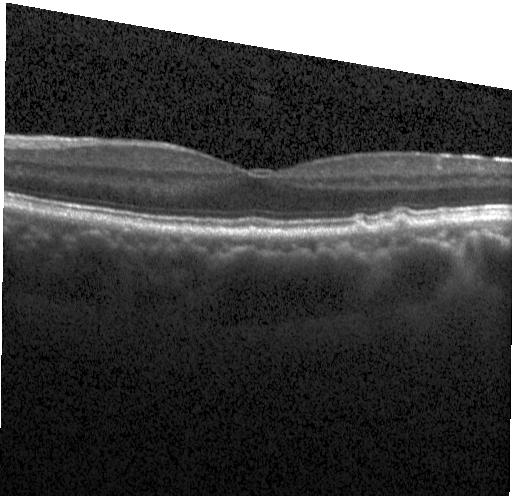
OCT line scan; centered on the fovea; Heidelberg Spectralis OCT system; spectral-domain optical coherence tomography — Finding: multiple drusen.